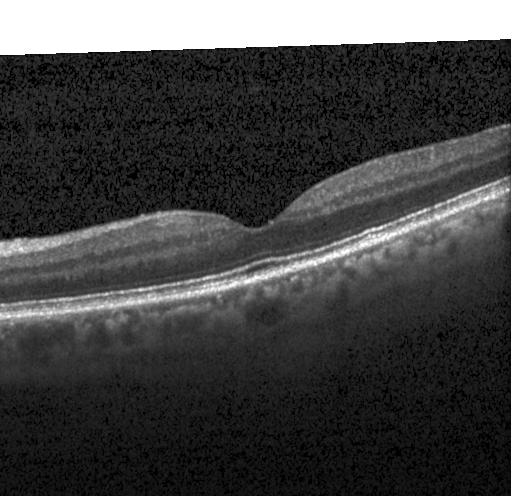
The scan shows neither choroidal neovascularization, diabetic macular edema, nor drusen.